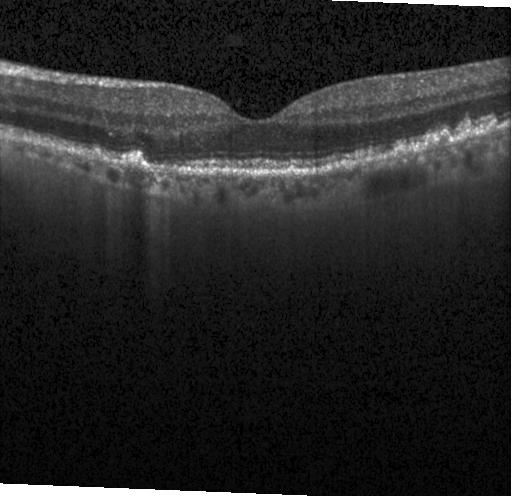

Retinal OCT B-scan
The scan shows sub-RPE drusenoid deposits.